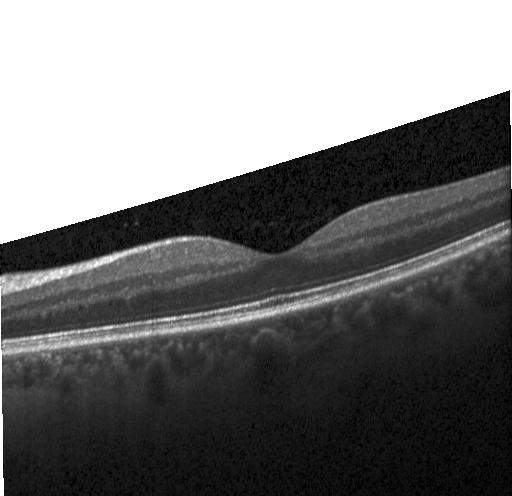 Macular scan; retinal OCT B-scan; spectral-domain OCT
Assessment: no evidence of choroidal neovascularization, diabetic macular edema, or drusen.